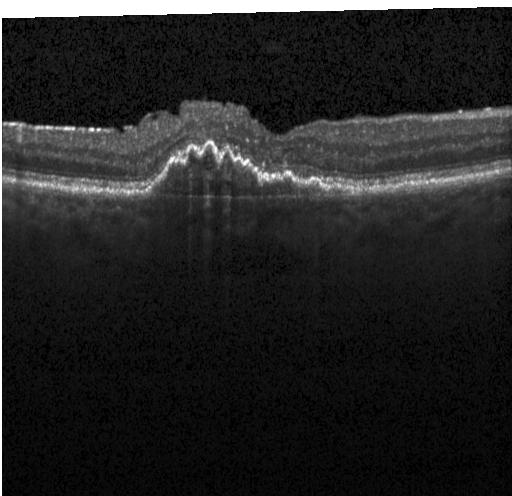 Acquired on a Heidelberg Spectralis · centered on the fovea · OCT line scan.
Diagnosis: a choroidal neovascular membrane.